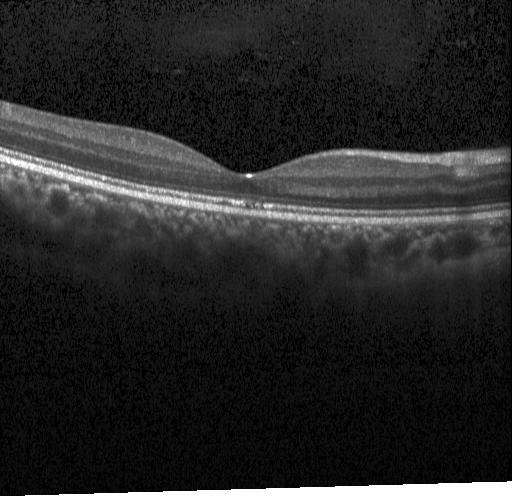

OCT B-scan. Centered on the fovea. Spectral-domain optical coherence tomography
Finding: no evidence of choroidal neovascularization, diabetic macular edema, or drusen.